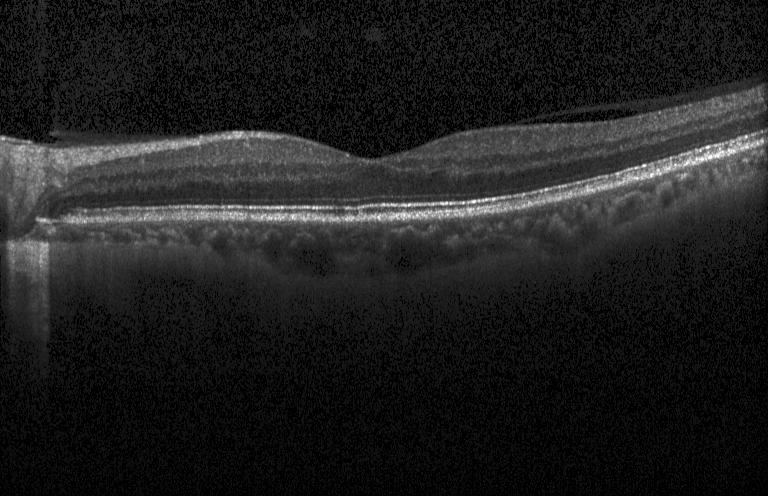

Retinal OCT B-scan, through the macula, instrument: Heidelberg Spectralis, spectral-domain OCT.
Diagnosis: no choroidal neovascularization, diabetic macular edema, or drusen.